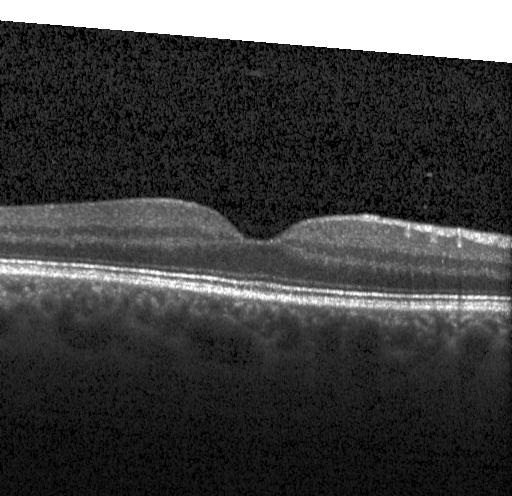
Macular OCT: neither CNV, DME, nor drusen.